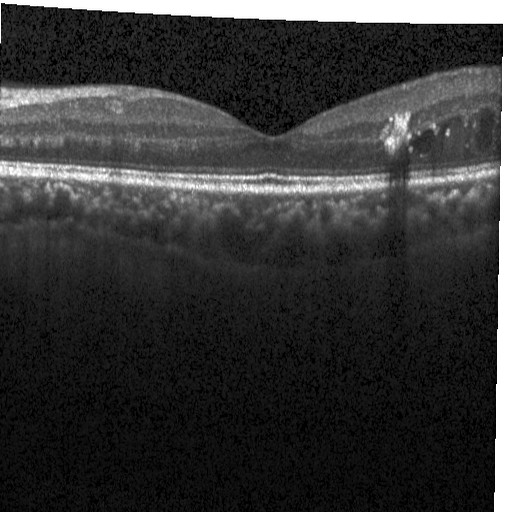 Optical coherence tomography B-scan · macular scan · spectral-domain OCT — Finding: diabetic macular edema.